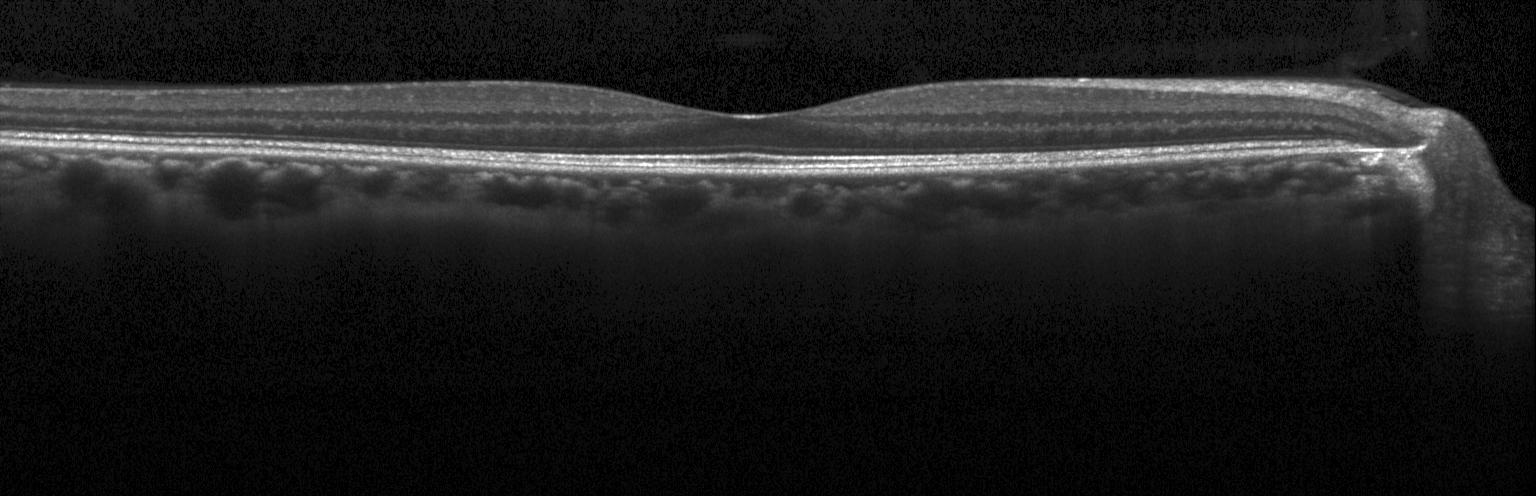

Macular OCT demonstrating neither CNV, DME, nor drusen.